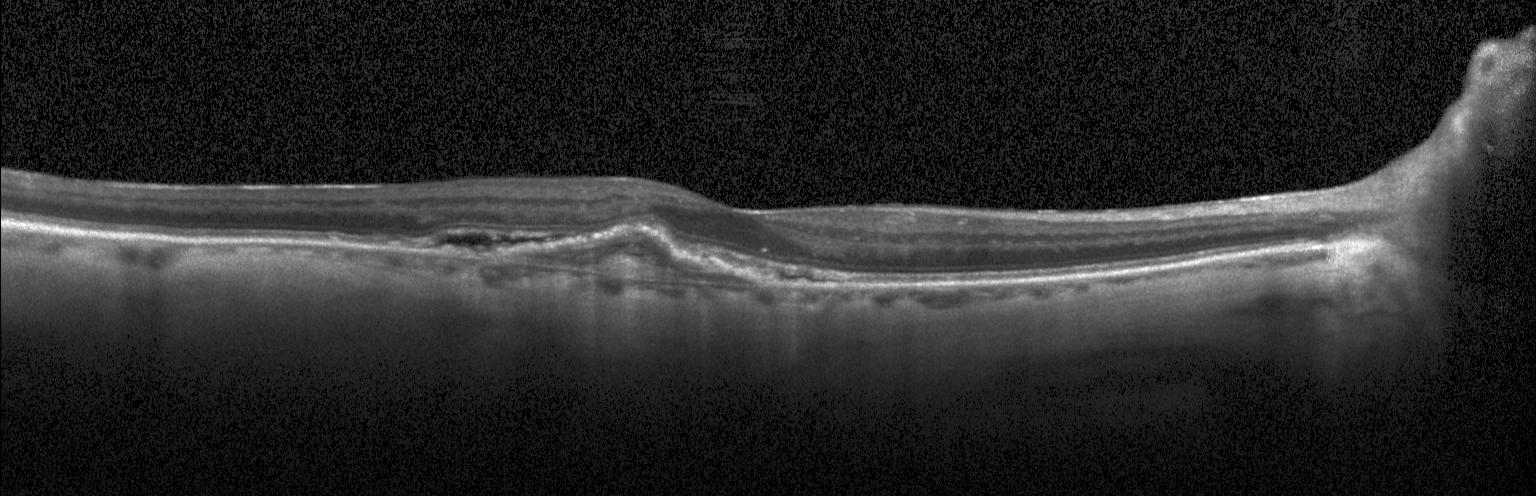
Spectral-domain optical coherence tomography; OCT line scan — Diagnosis: a choroidal neovascular membrane.